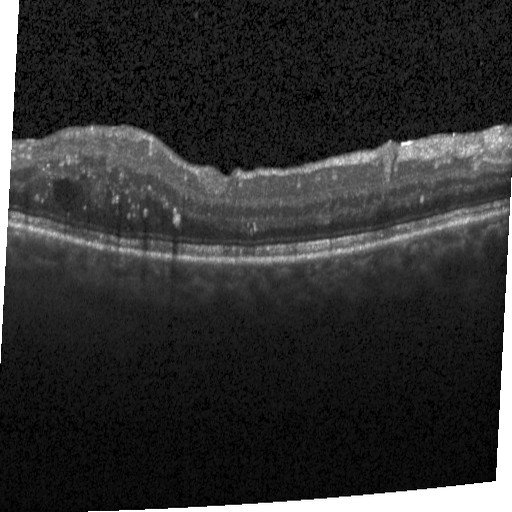 OCT B-scan showing diabetic macular edema (DME).